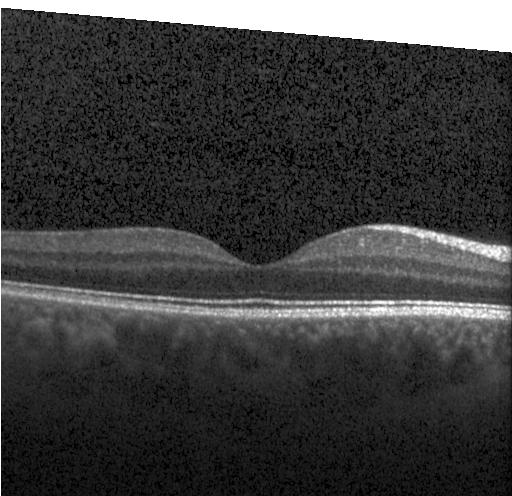

Macular OCT demonstrating no CNV, DME, or drusen.